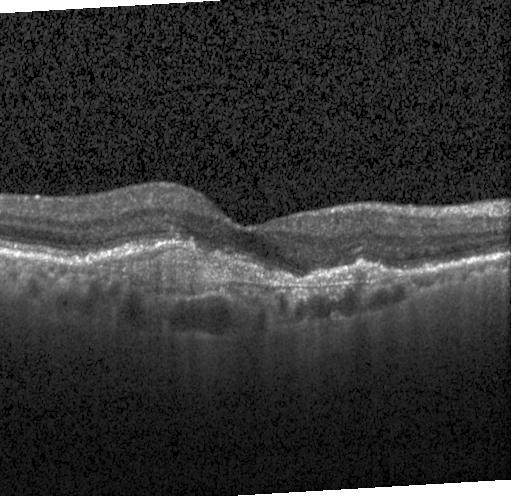

Macular OCT: a choroidal neovascular membrane.